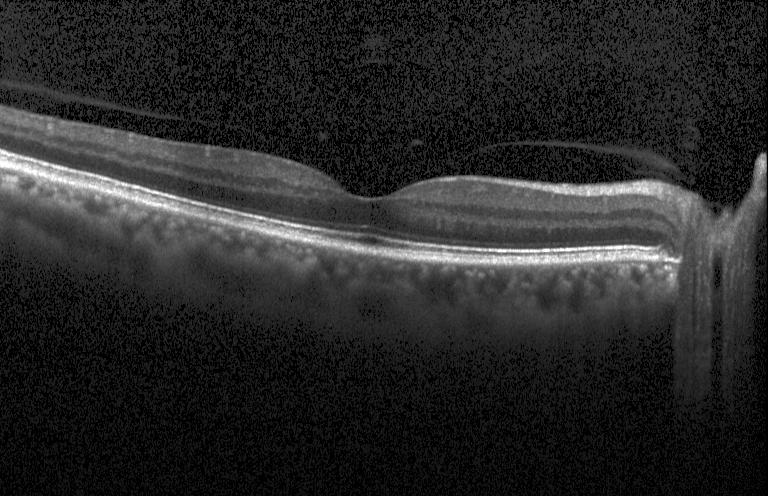 Retinal OCT cross-section.
The scan shows neither choroidal neovascularization, diabetic macular edema, nor drusen.